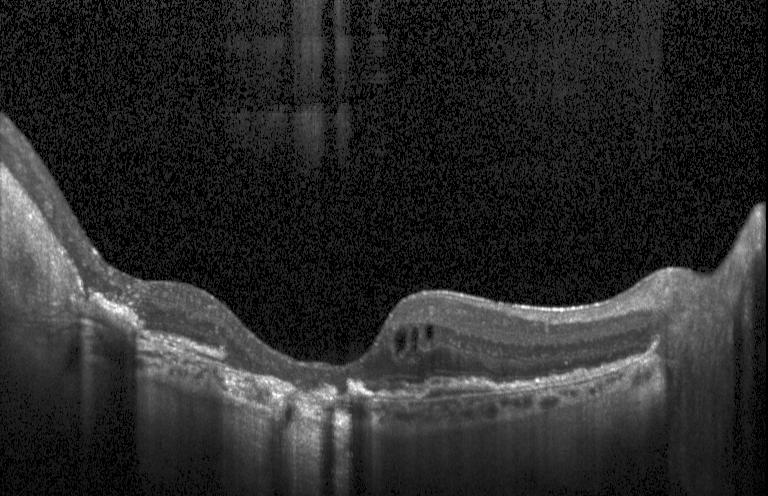 Impression: a choroidal neovascular membrane.